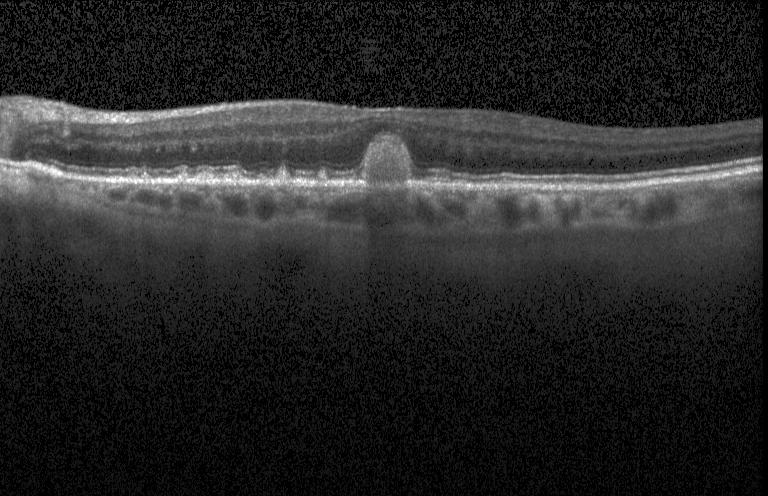
Diagnosis: choroidal neovascularization.